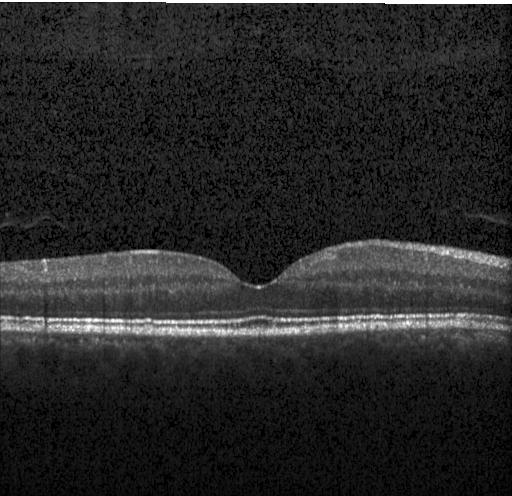
Dx: no evidence of choroidal neovascularization, diabetic macular edema, or drusen.